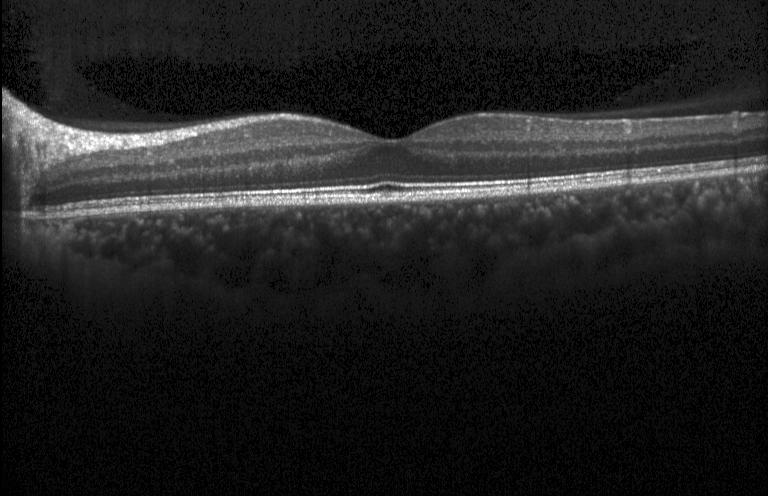

Diagnosis: neither choroidal neovascularization, diabetic macular edema, nor drusen.